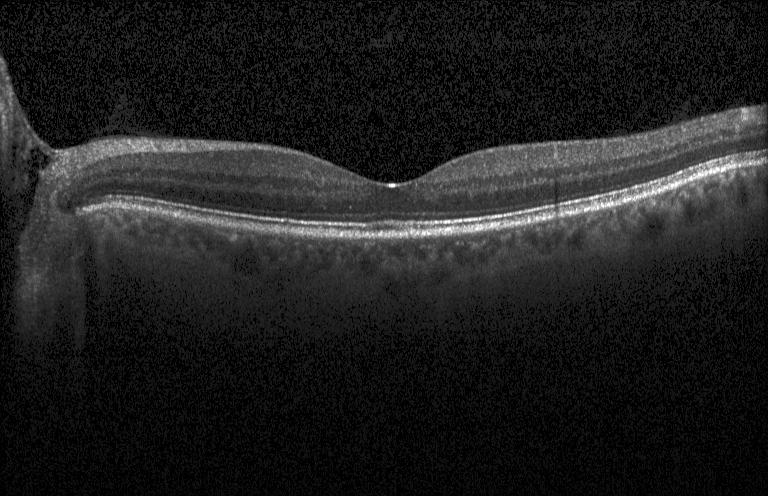 OCT scan showing no choroidal neovascularization, diabetic macular edema, or drusen.